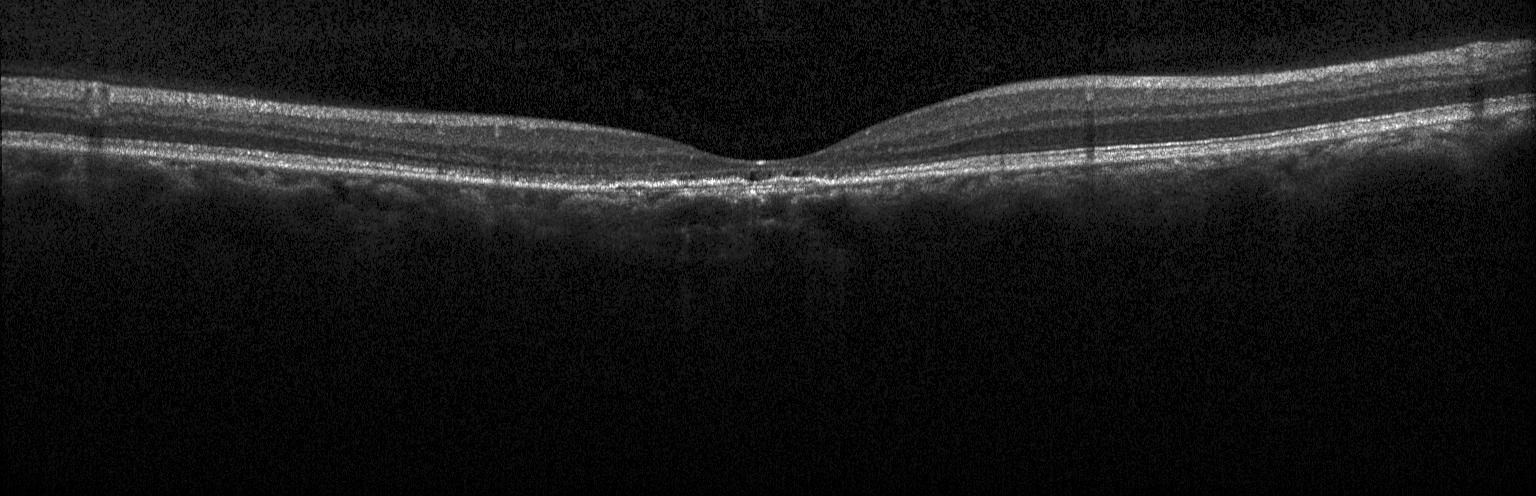
Impression: CNV.